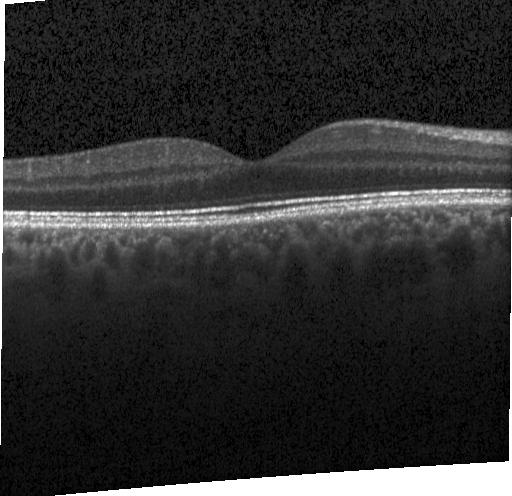
Spectral-domain optical coherence tomography. Optical coherence tomography B-scan.
Macular OCT: neither choroidal neovascularization, diabetic macular edema, nor drusen.